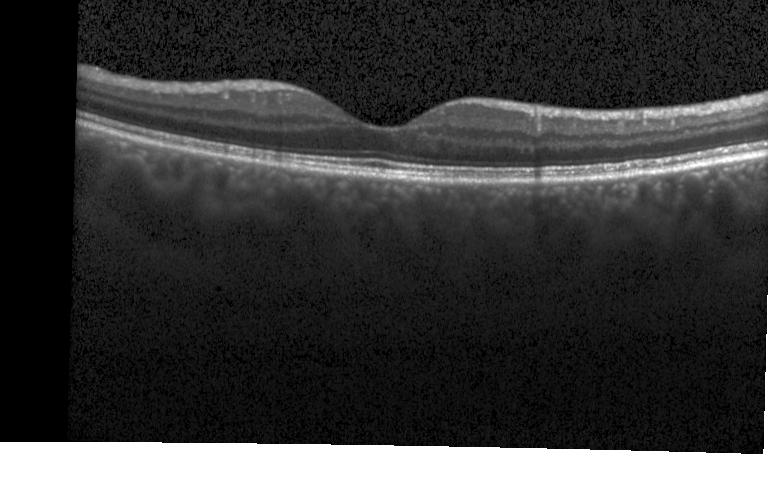
Macular OCT: no evidence of choroidal neovascularization, diabetic macular edema, or drusen.